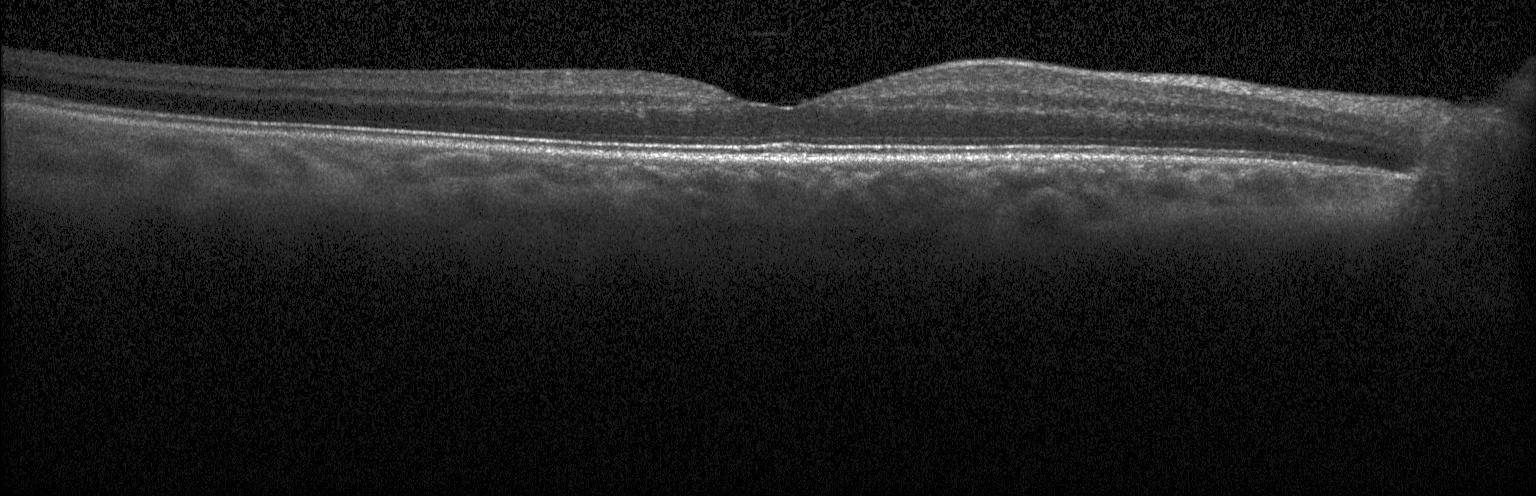 Macular OCT demonstrating no choroidal neovascularization, diabetic macular edema, or drusen.